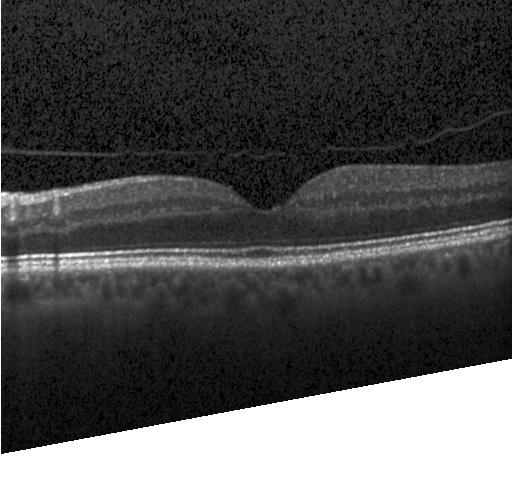 Fovea-centered, optical coherence tomography scan — Impression: no CNV, DME, or drusen.